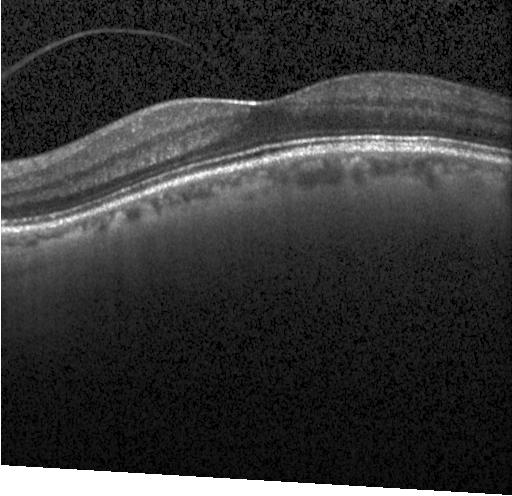

OCT B-scan showing no choroidal neovascularization, diabetic macular edema, or drusen.